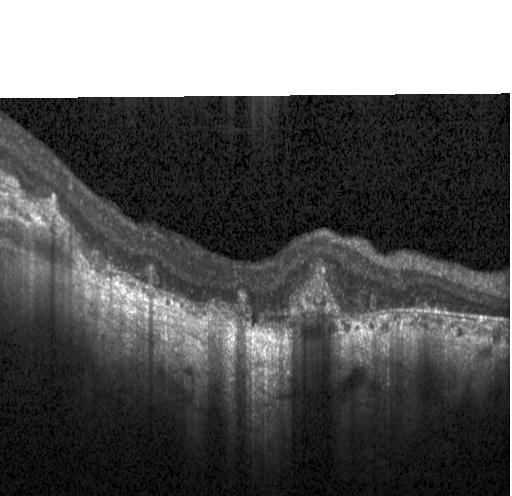
Optical coherence tomography B-scan, acquired on a Heidelberg Spectralis, macular scan, spectral-domain OCT — Choroidal neovascularization (CNV).